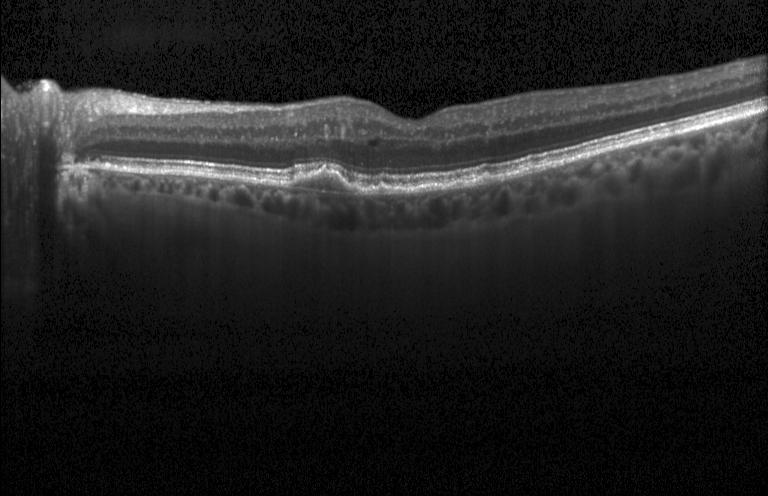
SD-OCT. Heidelberg Spectralis. Horizontal scan through the fovea. Retinal OCT cross-section — Assessment: a choroidal neovascular membrane.